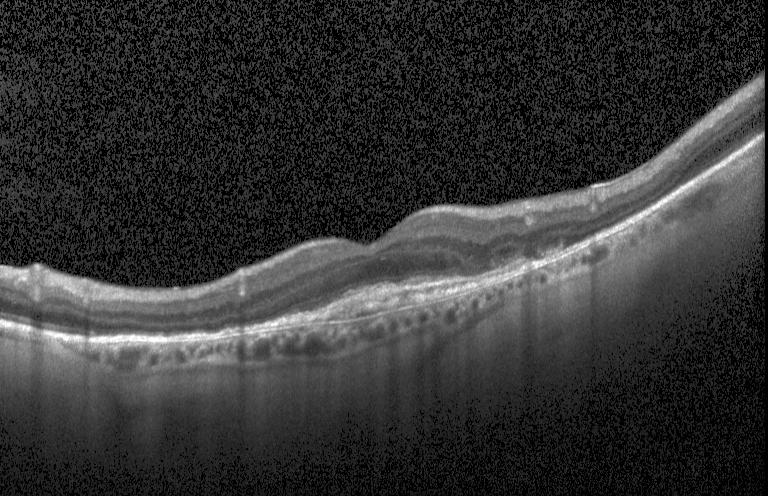 Horizontal scan through the fovea · retinal OCT B-scan
Macular OCT: CNV.